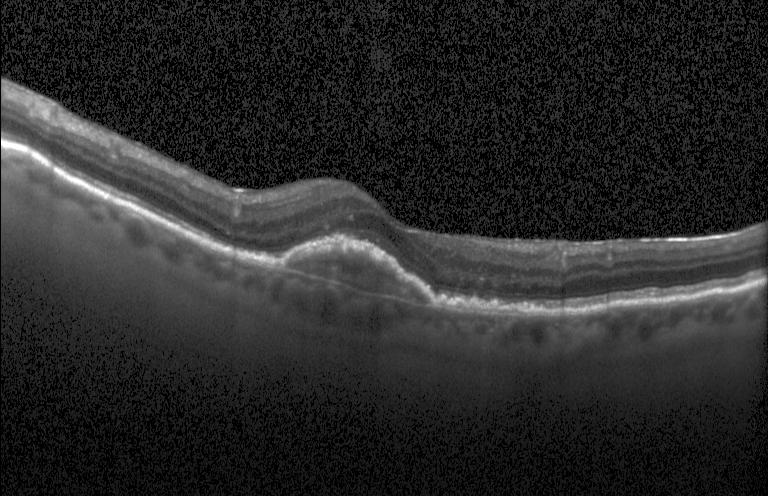

Macular OCT: choroidal neovascularization (CNV).